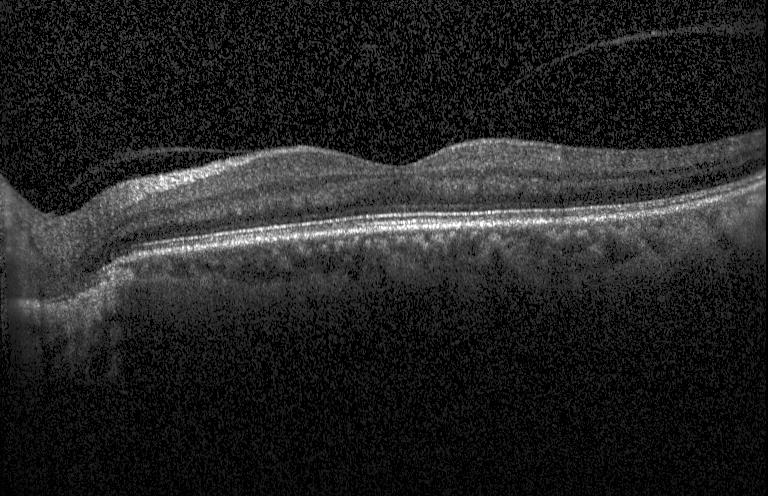 Optical coherence tomography scan · SD-OCT · fovea-centered — No choroidal neovascularization, no diabetic macular edema, and no drusen.